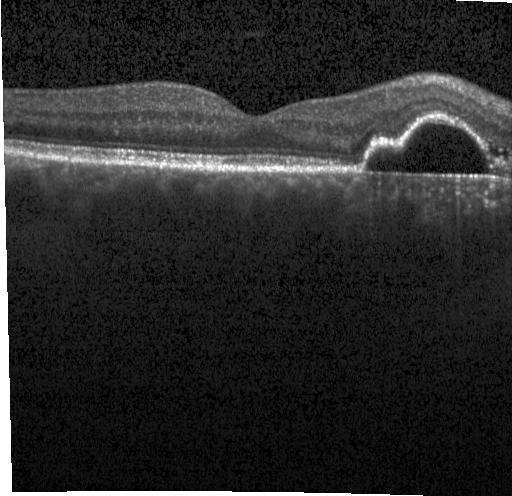

Macular OCT: CNV.